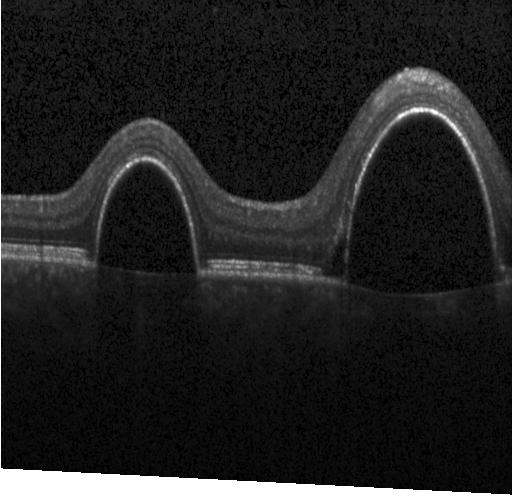 OCT scan showing choroidal neovascularization (CNV).